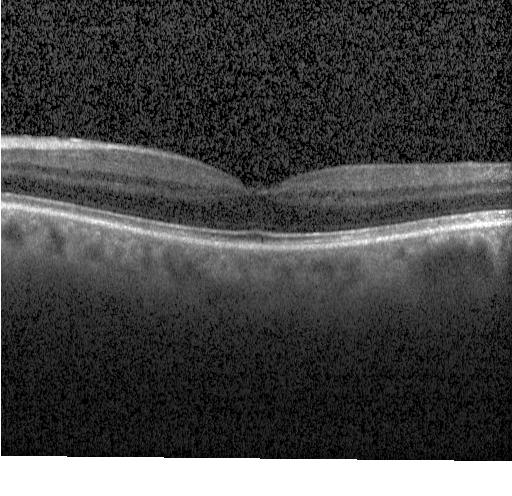
Retinal OCT cross-section showing no evidence of CNV, DME, or drusen.